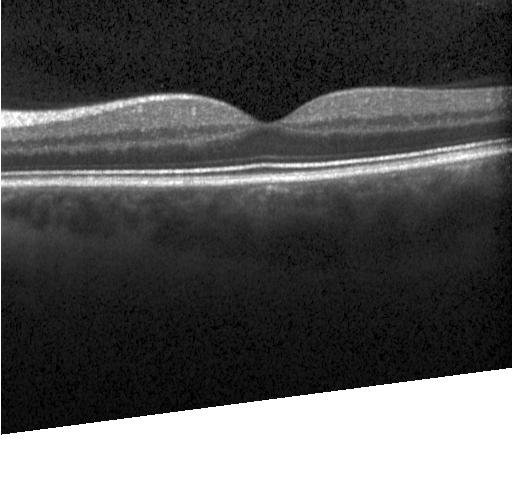 Spectral-domain optical coherence tomography. OCT B-scan.
OCT finding: no choroidal neovascularization, no diabetic macular edema, and no drusen.